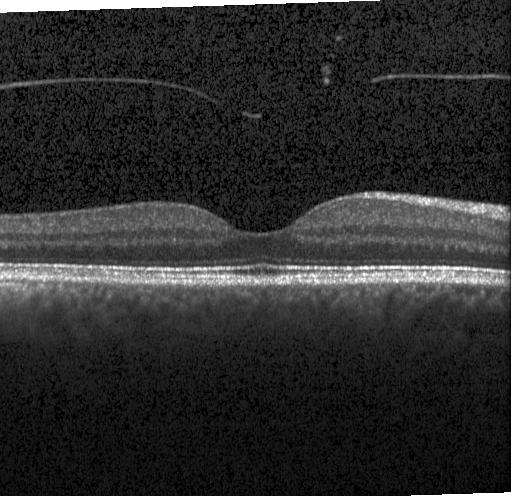
Dx: neither choroidal neovascularization, diabetic macular edema, nor drusen.